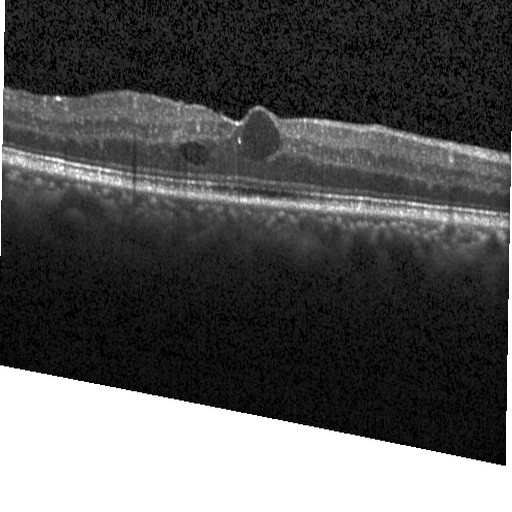
OCT B-scan showing diabetic macular edema (DME).